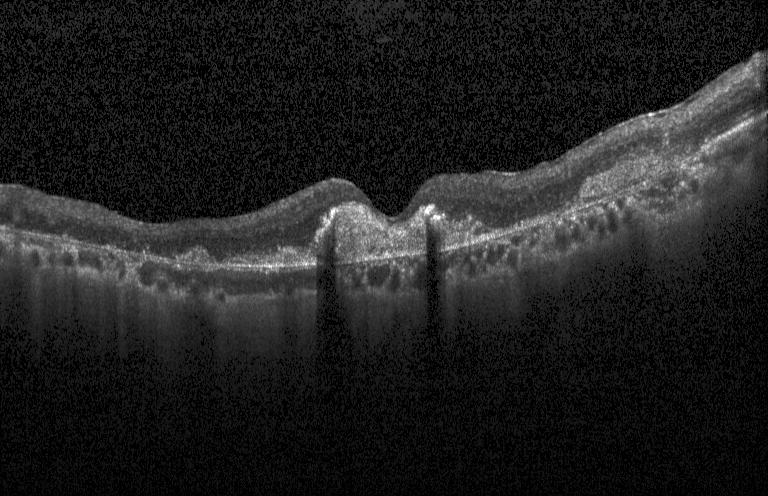

Diagnosis: a choroidal neovascular membrane.